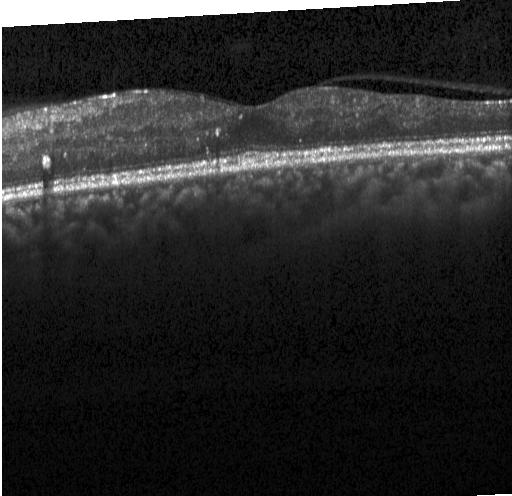 OCT line scan. Finding: diabetic macular edema.